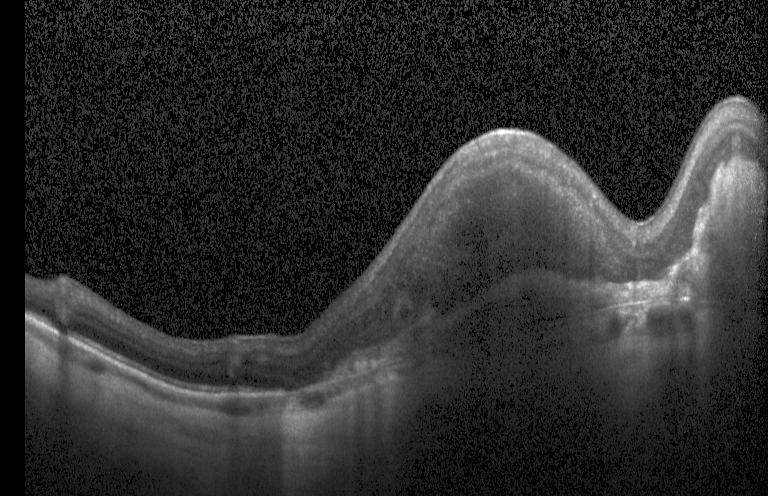 Optical coherence tomography scan; through the macula; SD-OCT; instrument: Heidelberg Spectralis. Finding: a choroidal neovascular membrane.